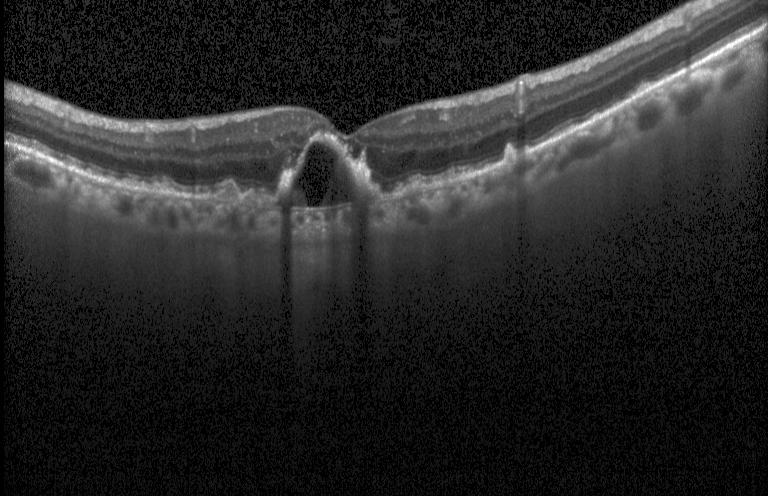
A choroidal neovascular membrane.